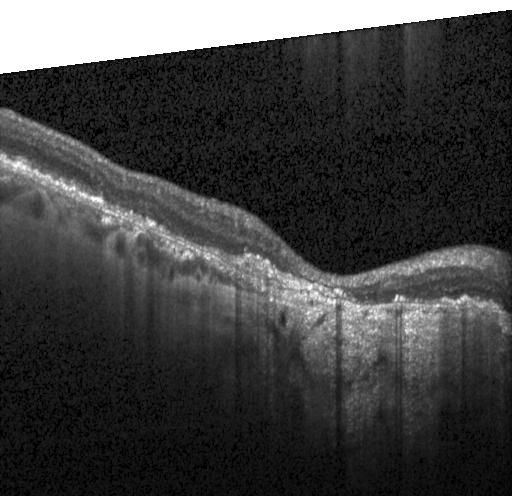
OCT line scan · spectral-domain OCT · acquired on a Heidelberg Spectralis. Choroidal neovascularization (CNV).